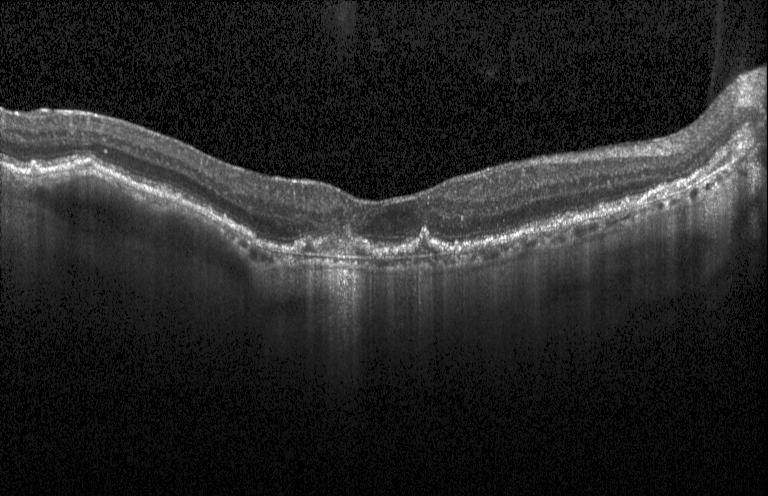
Dx: choroidal neovascularization.